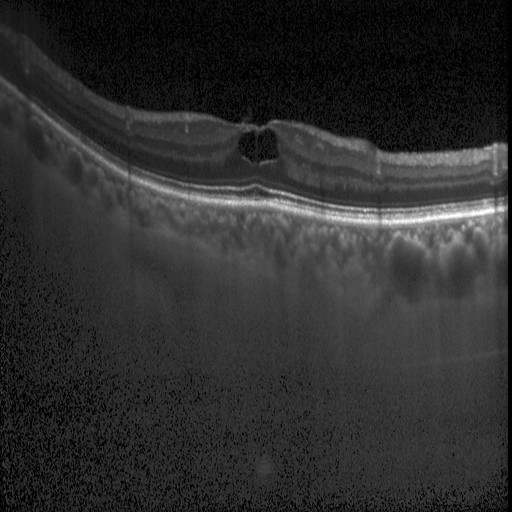 Fovea-centered. SD-OCT. OCT B-scan. Finding: diabetic macular edema (DME).